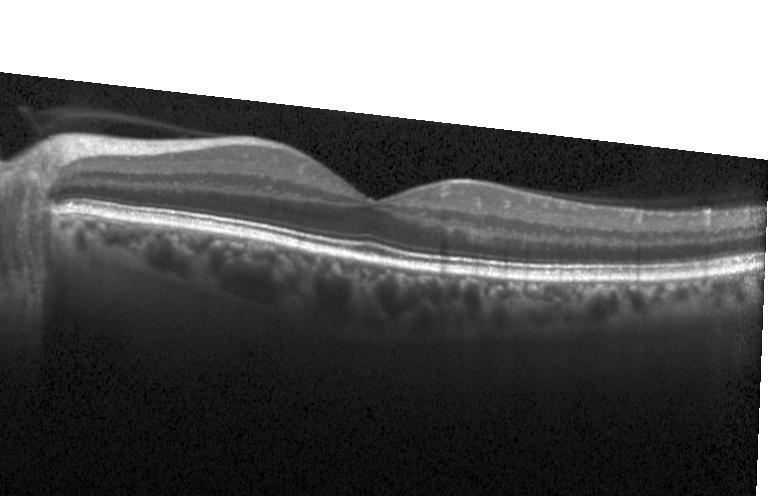
OCT line scan, Heidelberg Spectralis — Impression: no choroidal neovascularization, no diabetic macular edema, and no drusen.